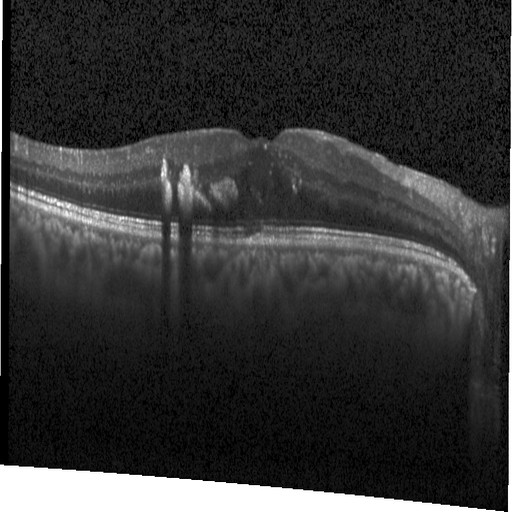 OCT B-scan; horizontal scan through the fovea; SD-OCT; acquired on a Heidelberg Spectralis. Macular OCT: diabetic macular edema.